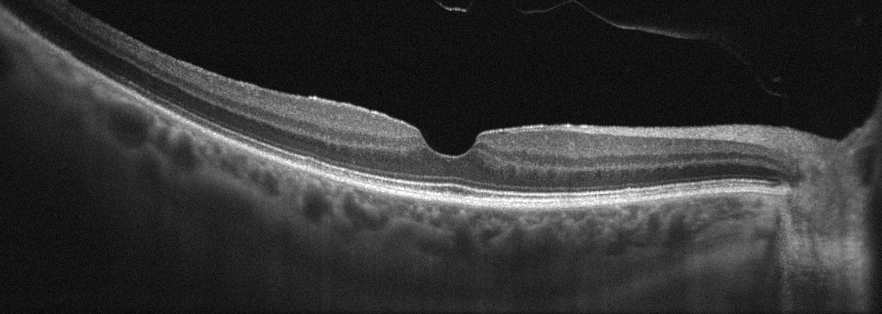
OCT line scan · right eye
Epiretinal membrane.